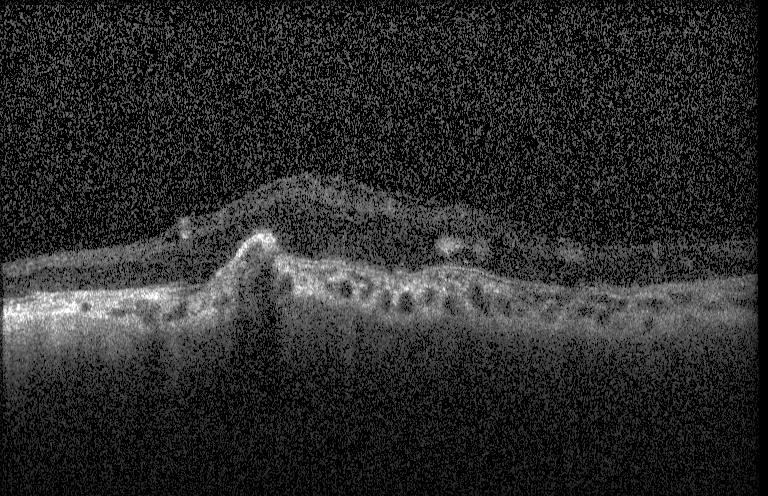 Diagnosis: a choroidal neovascular membrane.